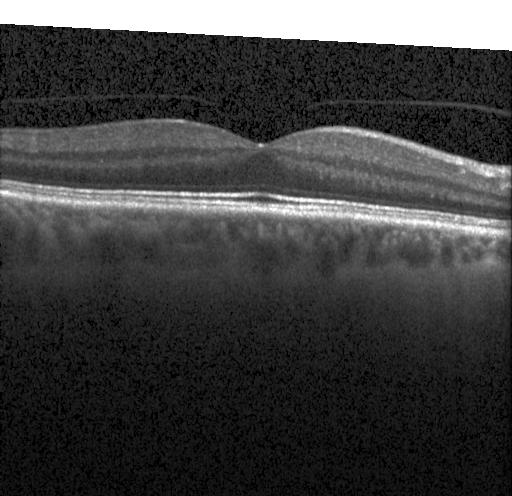 Heidelberg Spectralis, OCT B-scan, spectral-domain OCT — Assessment: no choroidal neovascularization, diabetic macular edema, or drusen.